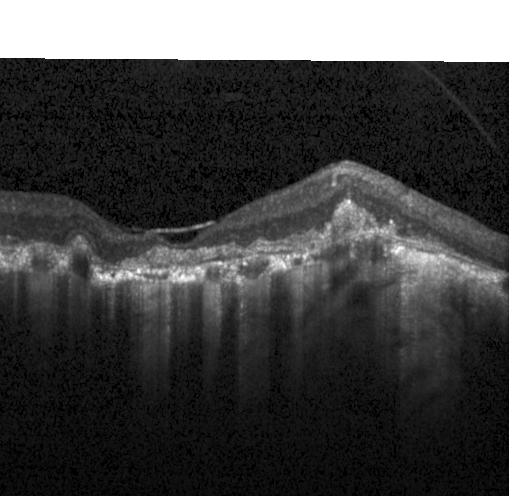 OCT B-scan, spectral-domain OCT
Macular OCT: choroidal neovascularization.